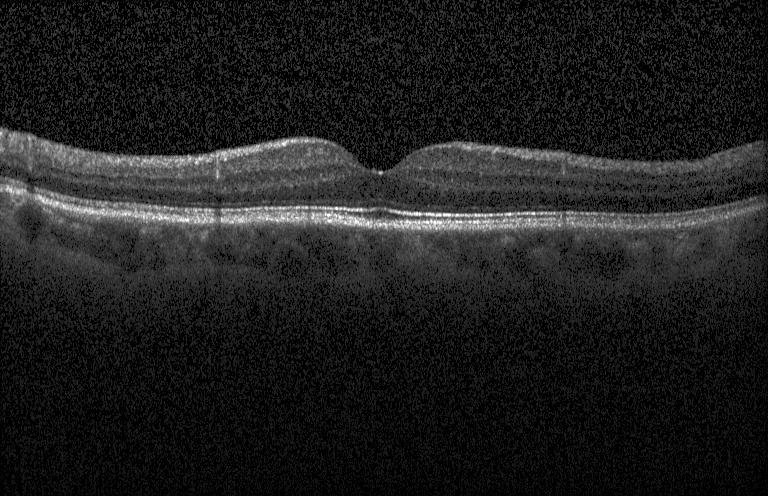

Impression: no CNV, DME, or drusen.